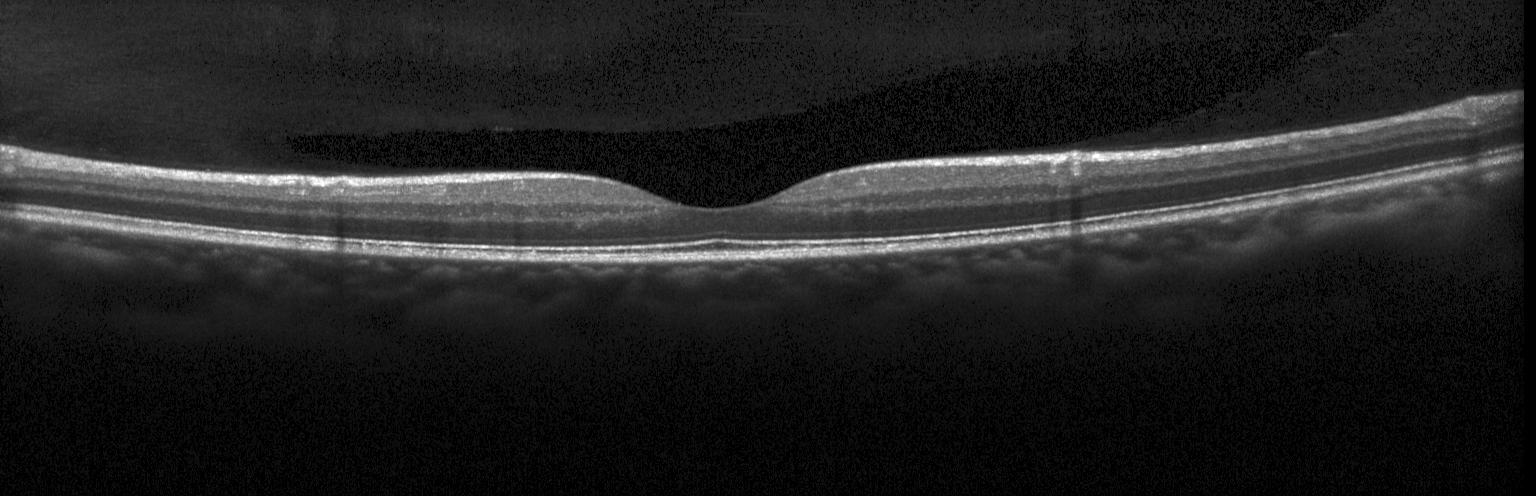
Macular OCT demonstrating no choroidal neovascularization, no diabetic macular edema, and no drusen.